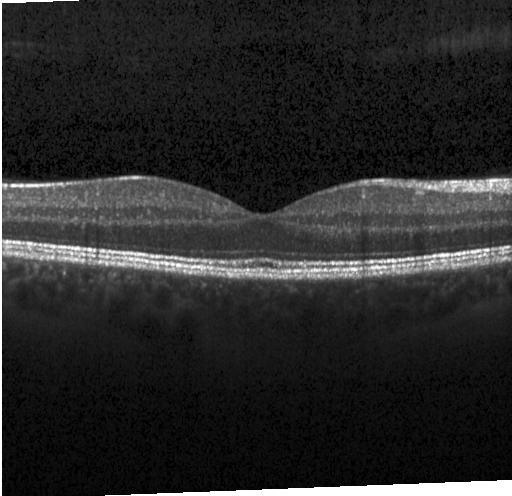 OCT line scan.
Diagnosis: no CNV, DME, or drusen.